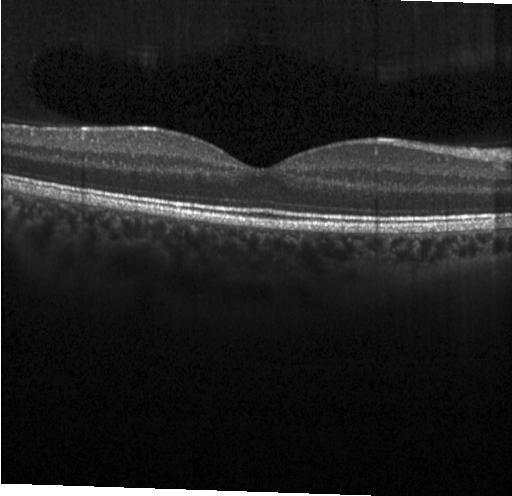
OCT B-scan.
Diagnosis: neither CNV, DME, nor drusen.